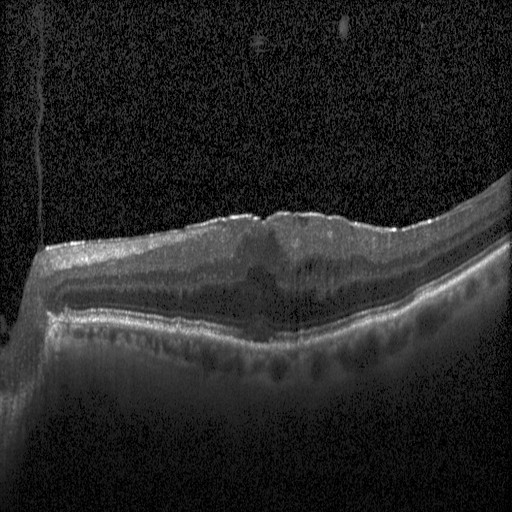 Spectral-domain OCT; OCT B-scan; through the macula; Heidelberg Spectralis OCT system
Diagnosis: diabetic macular edema.